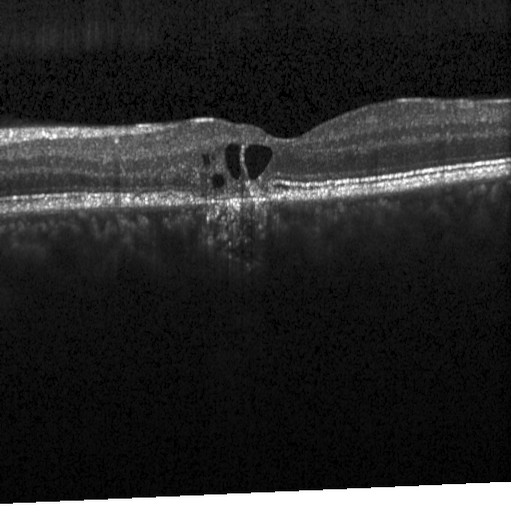

OCT B-scan. The scan shows diabetic macular edema (DME).